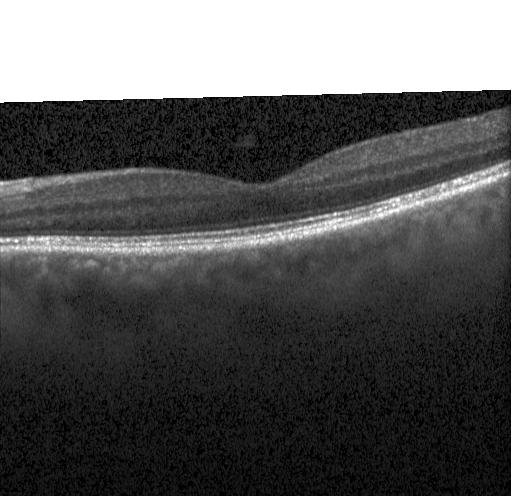

Instrument: Heidelberg Spectralis. Spectral-domain optical coherence tomography. Retinal OCT cross-section
Impression: no CNV, no DME, and no drusen.